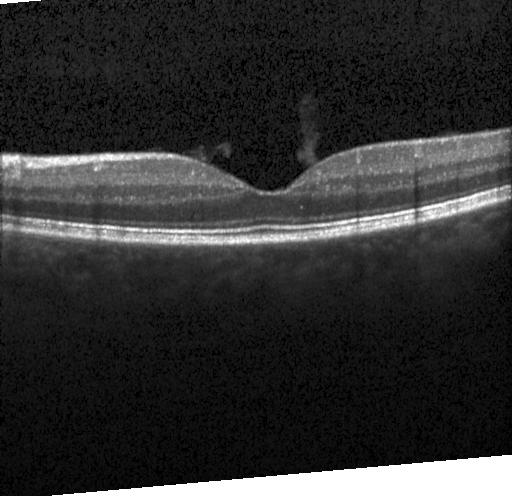 Neither choroidal neovascularization, diabetic macular edema, nor drusen.